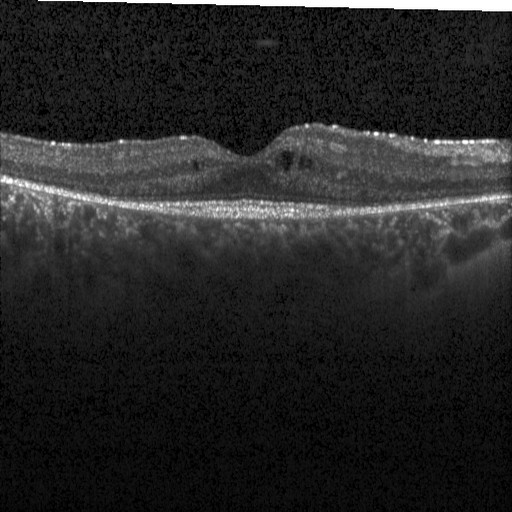
OCT B-scan.
This B-scan demonstrates DME.